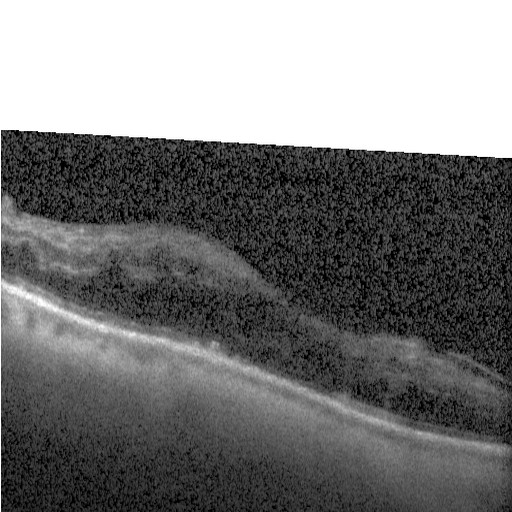
Finding: DME.